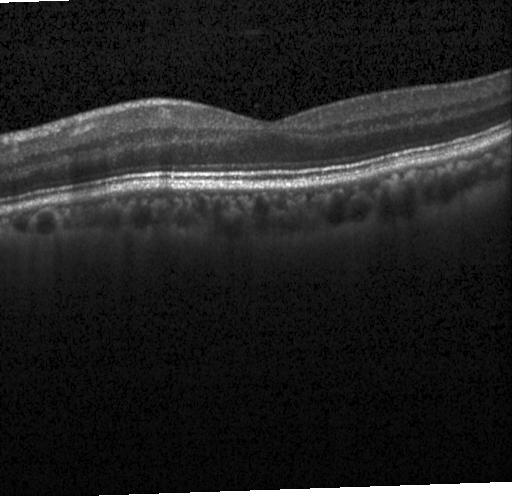

Retinal OCT cross-section; spectral-domain OCT
OCT finding: neither choroidal neovascularization, diabetic macular edema, nor drusen.